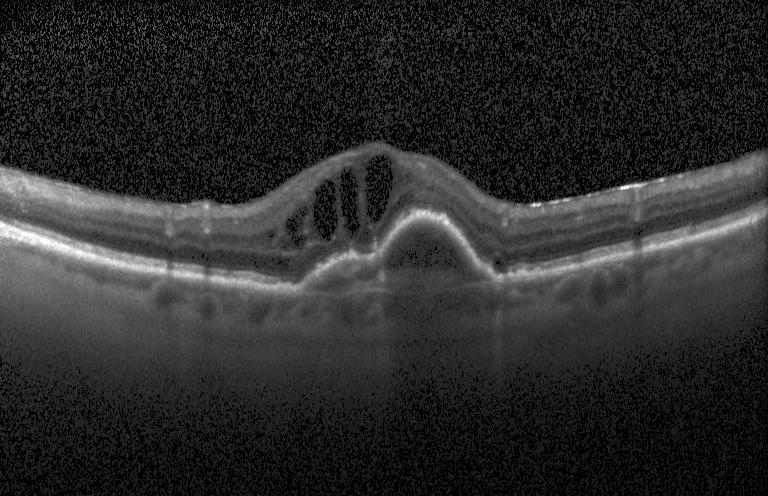

Optical coherence tomography B-scan · spectral-domain OCT. This B-scan demonstrates a choroidal neovascular membrane.